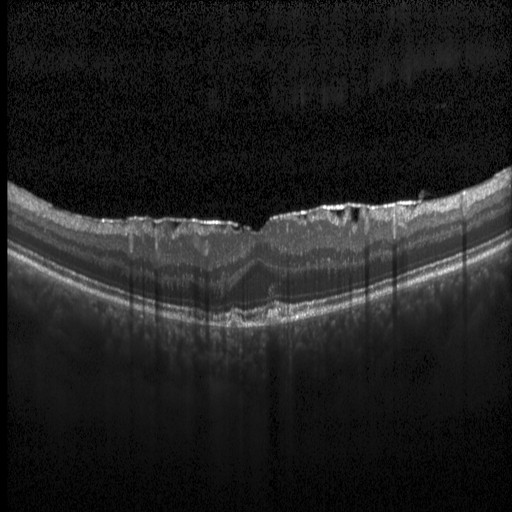

Heidelberg Spectralis OCT system, through the macula, OCT B-scan, spectral-domain OCT.
Finding: diabetic macular edema (DME).